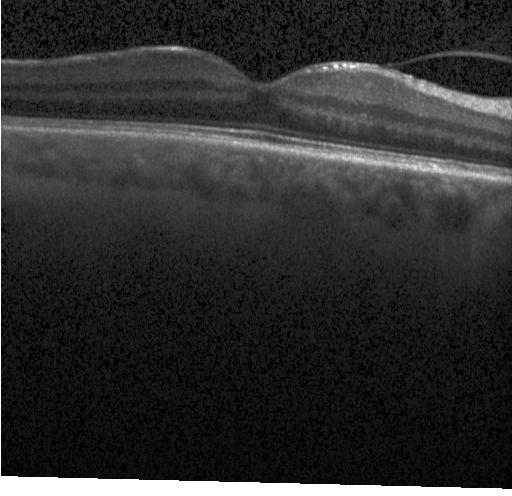

Retinal OCT cross-section, fovea-centered, spectral-domain optical coherence tomography. Impression: no CNV, DME, or drusen.